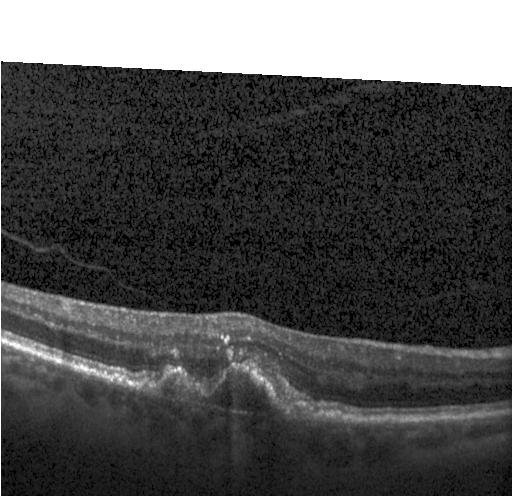
Macular OCT: CNV.